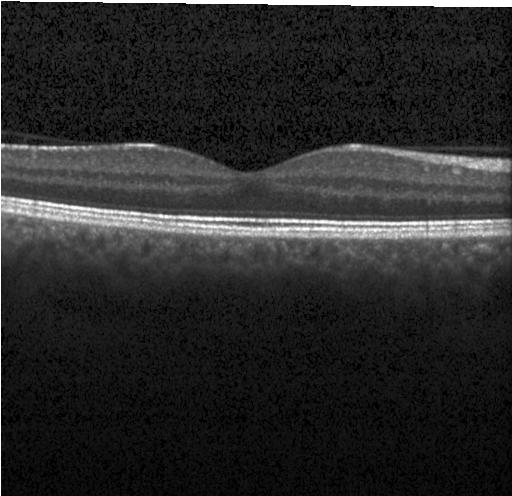 OCT finding: neither choroidal neovascularization, diabetic macular edema, nor drusen.